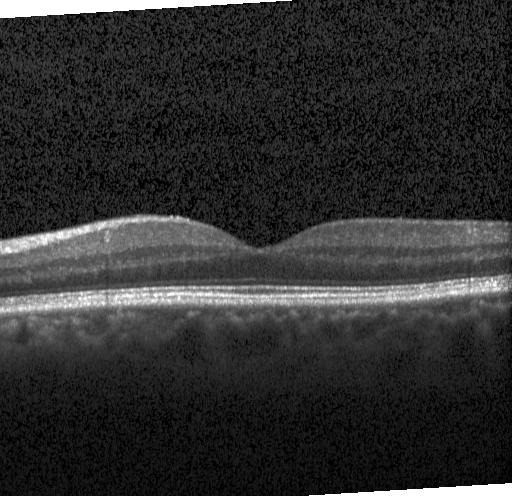
Spectral-domain optical coherence tomography; OCT line scan.
No evidence of CNV, DME, or drusen.